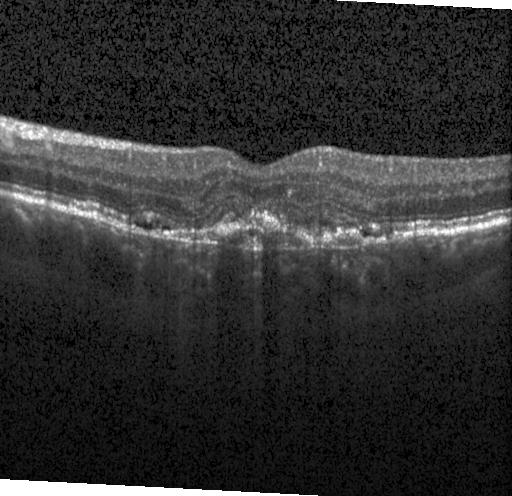

Retinal OCT cross-section showing choroidal neovascularization.